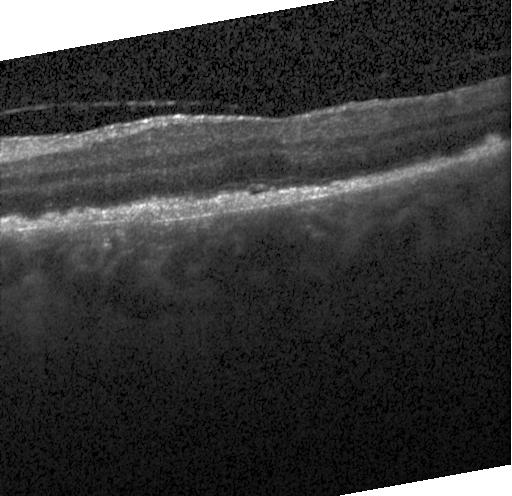

OCT B-scan showing choroidal neovascularization (CNV).